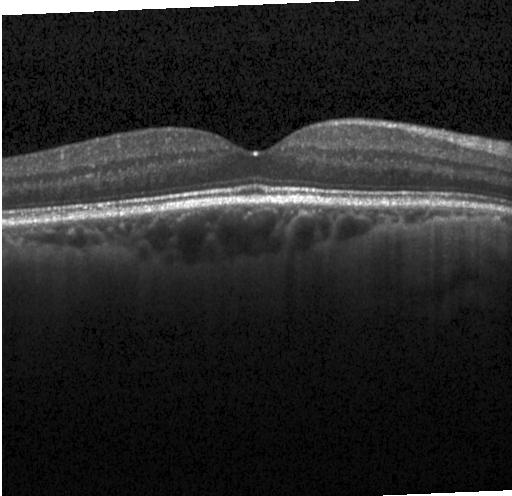
OCT B-scan showing no evidence of CNV, DME, or drusen.